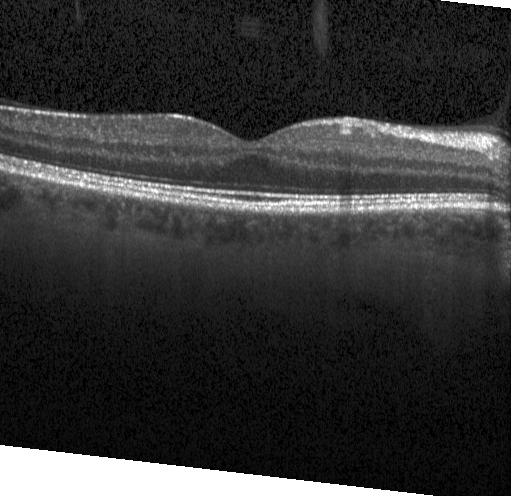 This B-scan demonstrates no choroidal neovascularization, no diabetic macular edema, and no drusen.